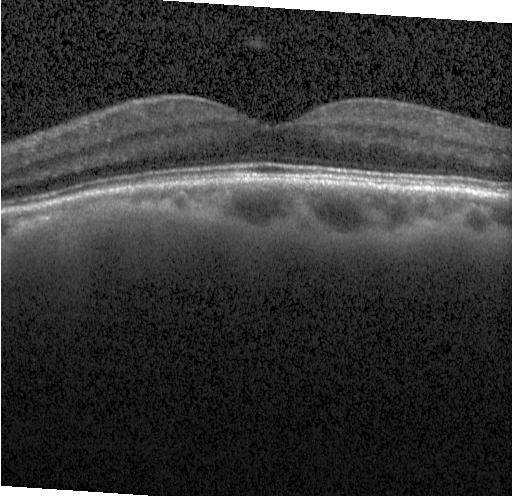 OCT finding: no choroidal neovascularization, no diabetic macular edema, and no drusen.